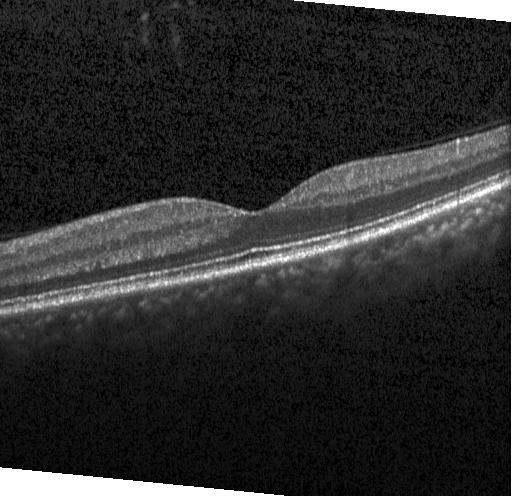
OCT B-scan, horizontal scan through the fovea. This B-scan demonstrates no choroidal neovascularization, no diabetic macular edema, and no drusen.